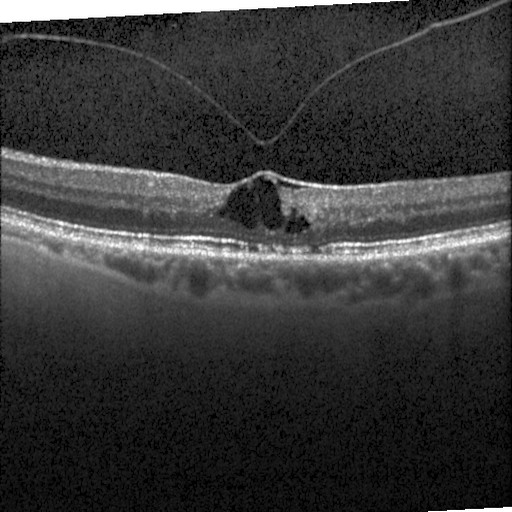 OCT line scan. This B-scan demonstrates DME.